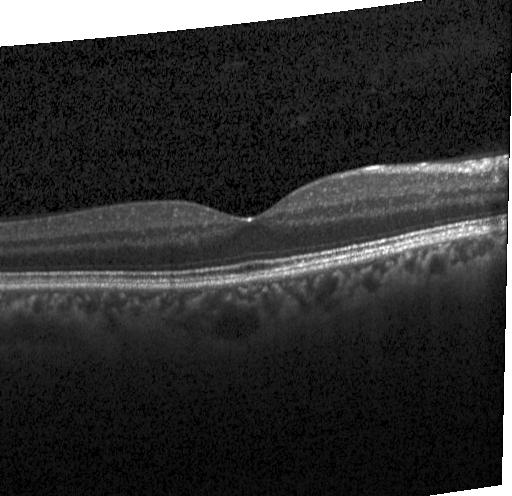

Impression: no CNV, no DME, and no drusen.